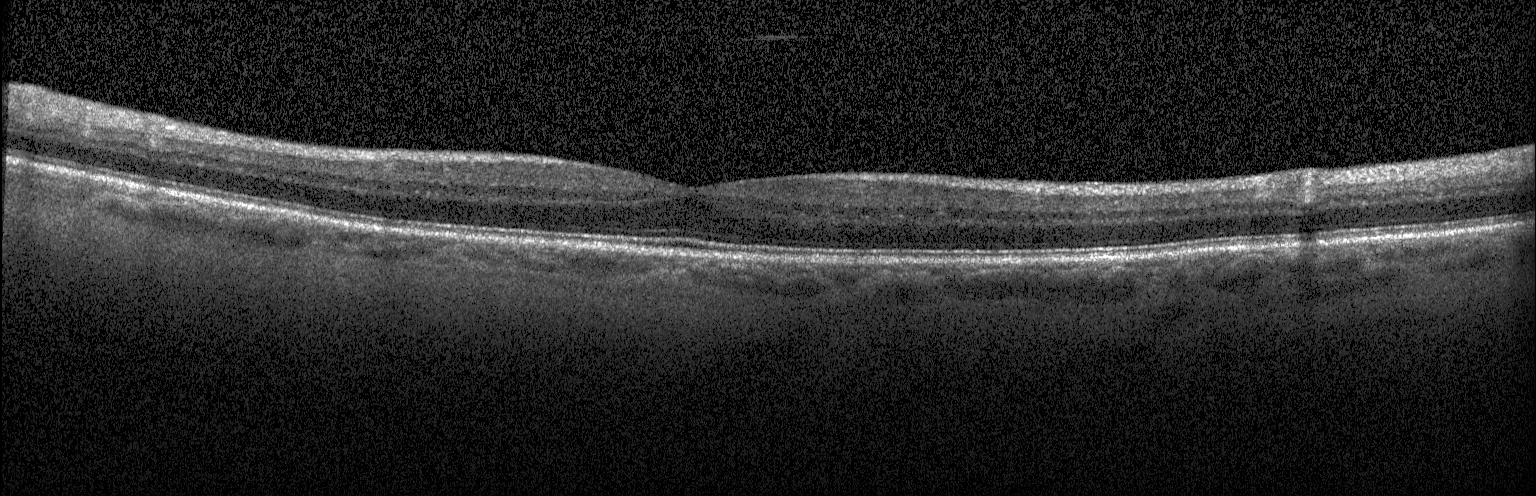 This B-scan demonstrates no evidence of choroidal neovascularization, diabetic macular edema, or drusen.